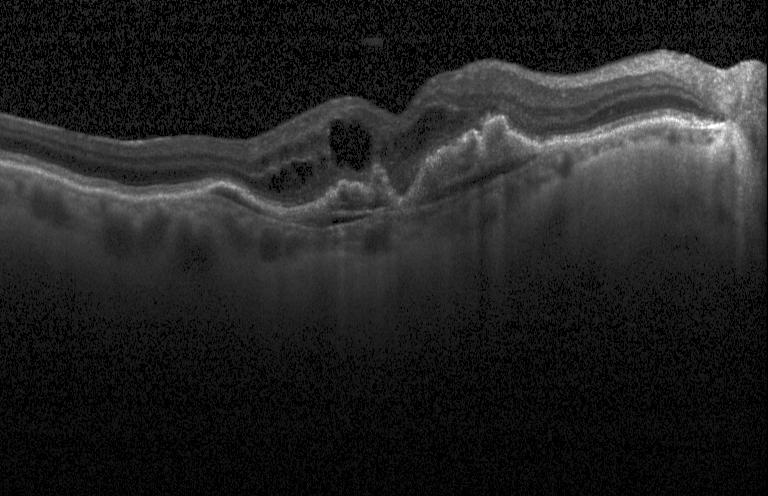 Horizontal scan through the fovea, OCT B-scan, spectral-domain optical coherence tomography
OCT finding: CNV.